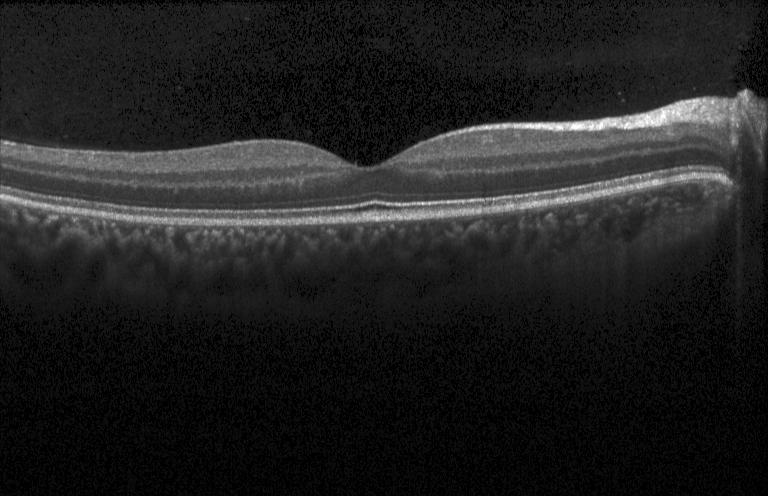
Optical coherence tomography scan
Finding: no CNV, DME, or drusen.